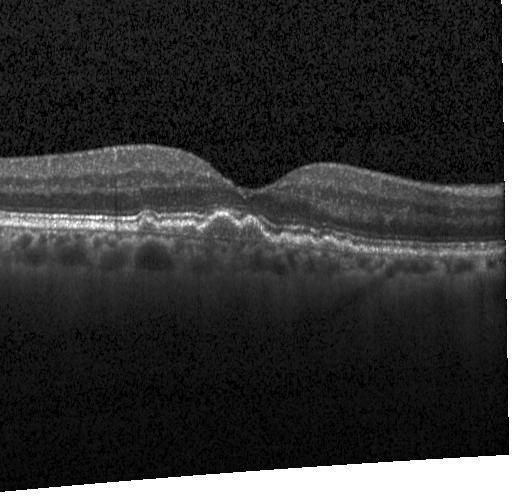 Retinal OCT B-scan. This B-scan demonstrates sub-RPE drusenoid deposits.